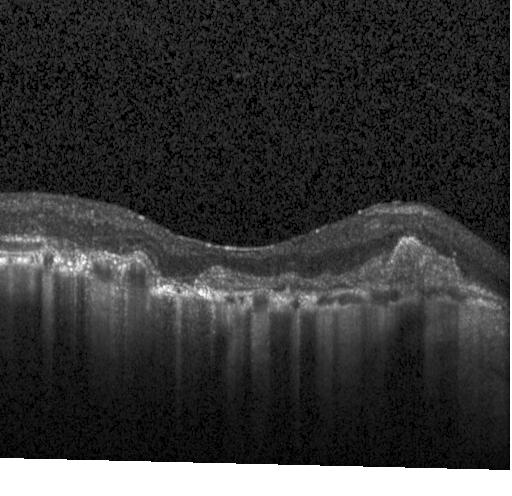 Diagnosis: CNV.